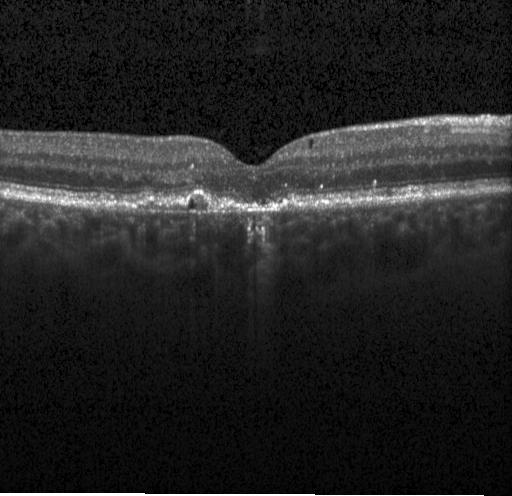 This B-scan demonstrates a choroidal neovascular membrane.